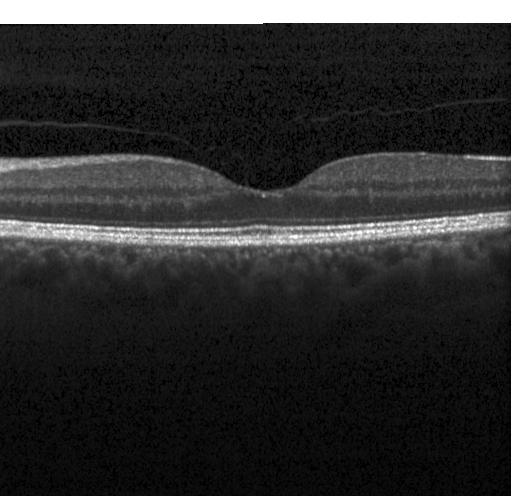 Macular OCT: no CNV, DME, or drusen.